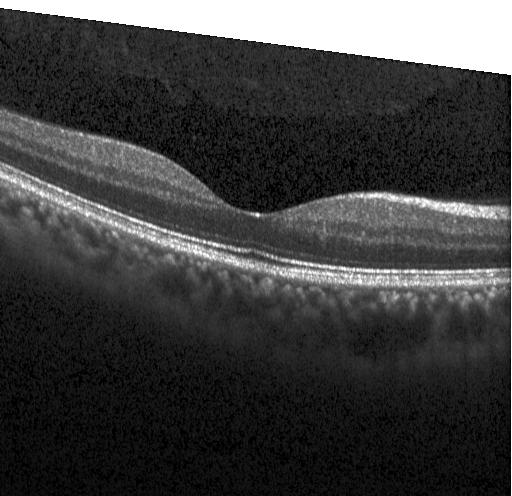
Heidelberg Spectralis, retinal OCT cross-section. Finding: no choroidal neovascularization, no diabetic macular edema, and no drusen.